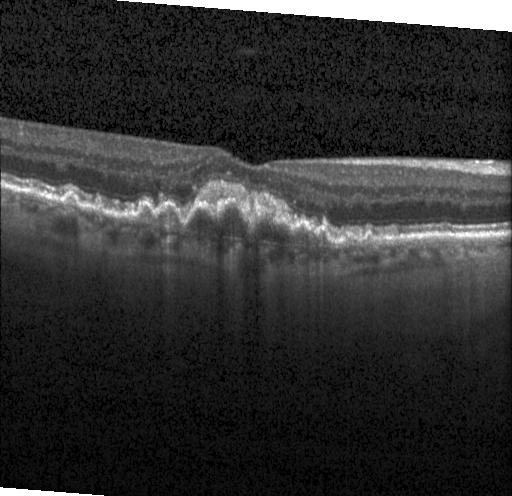 Optical coherence tomography scan — Assessment: a choroidal neovascular membrane.